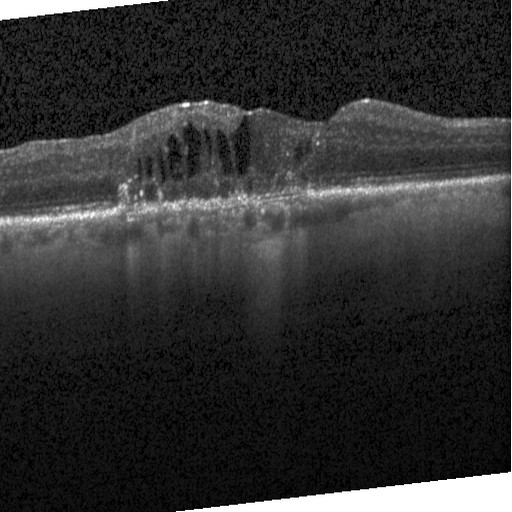

OCT line scan · fovea-centered. Impression: DME.